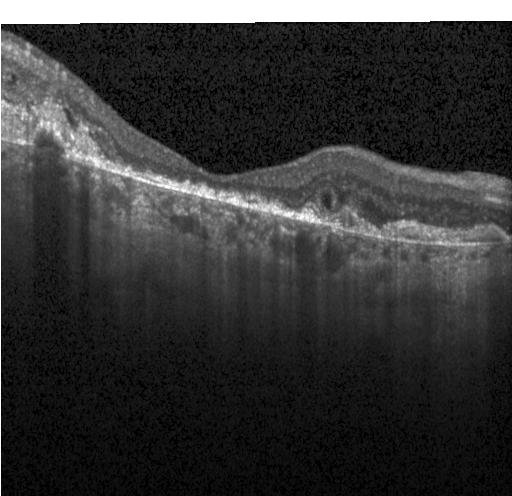 Impression: choroidal neovascularization (CNV).